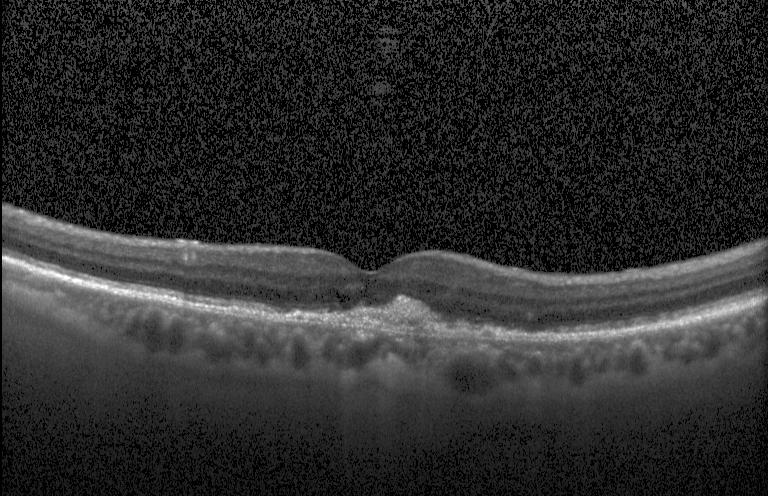
OCT B-scan showing CNV.